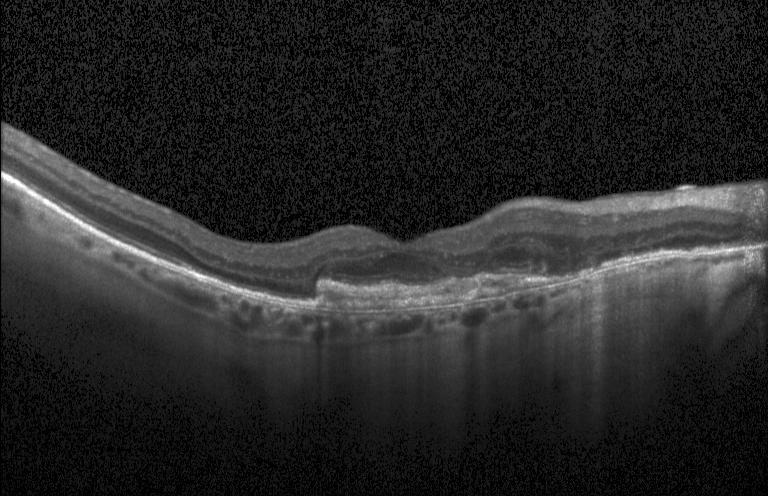

OCT B-scan, Heidelberg Spectralis OCT system.
This B-scan demonstrates a choroidal neovascular membrane.